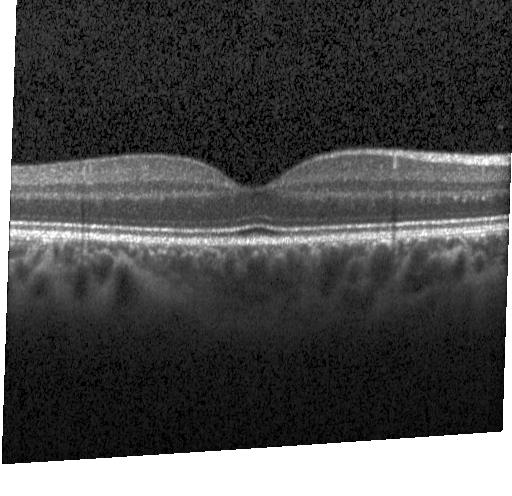
Optical coherence tomography scan
Diagnosis: no evidence of choroidal neovascularization, diabetic macular edema, or drusen.